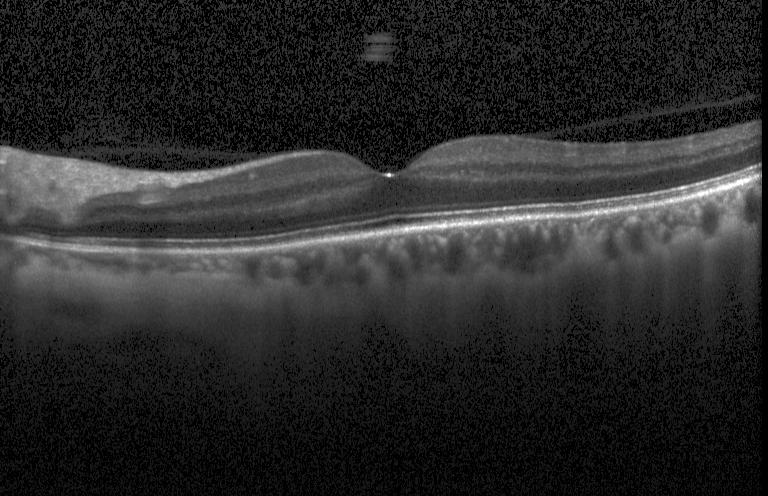

OCT scan showing no evidence of CNV, DME, or drusen.